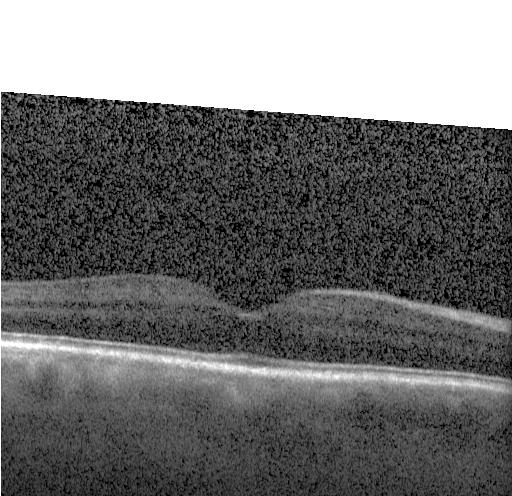

Spectral-domain OCT. Optical coherence tomography scan. Through the macula. Heidelberg Spectralis. The scan shows neither CNV, DME, nor drusen.